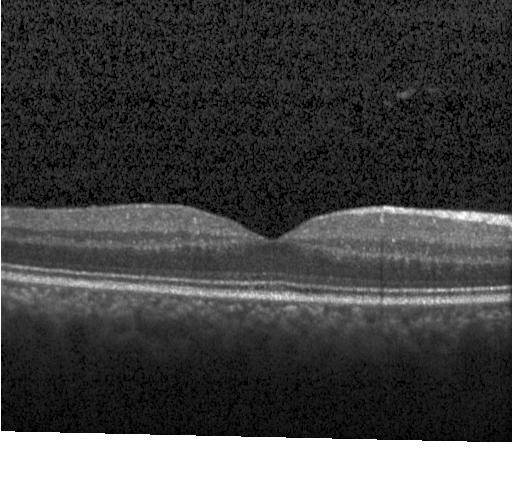 Optical coherence tomography scan, instrument: Heidelberg Spectralis, centered on the fovea
Macular OCT: no choroidal neovascularization, diabetic macular edema, or drusen.